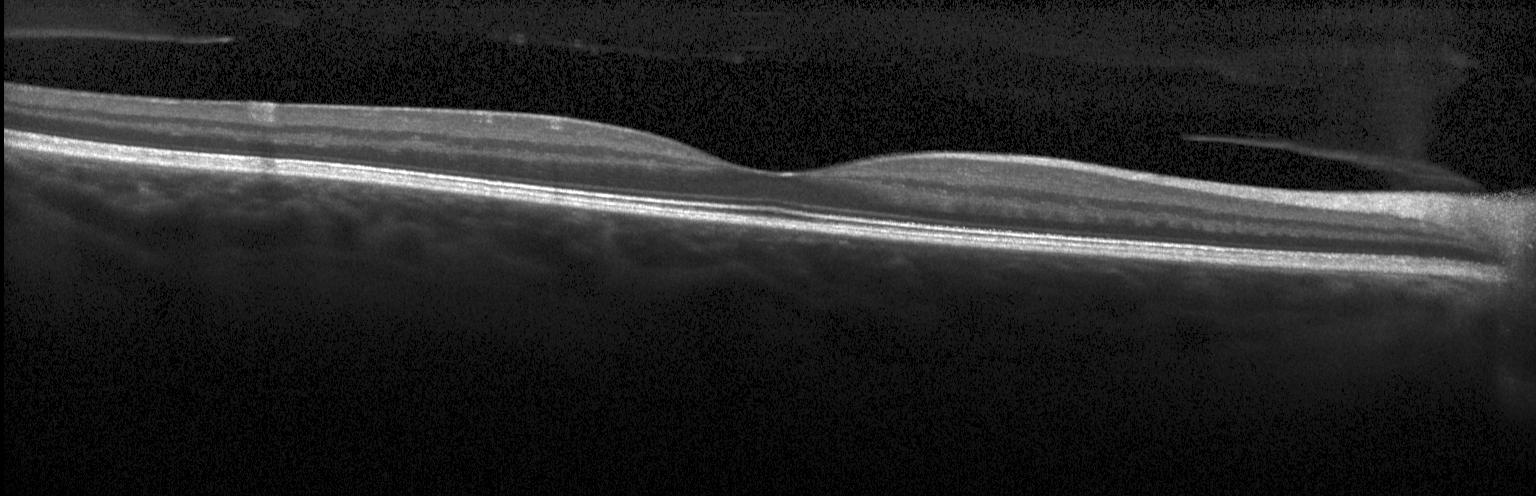

Diagnosis: no choroidal neovascularization, no diabetic macular edema, and no drusen.